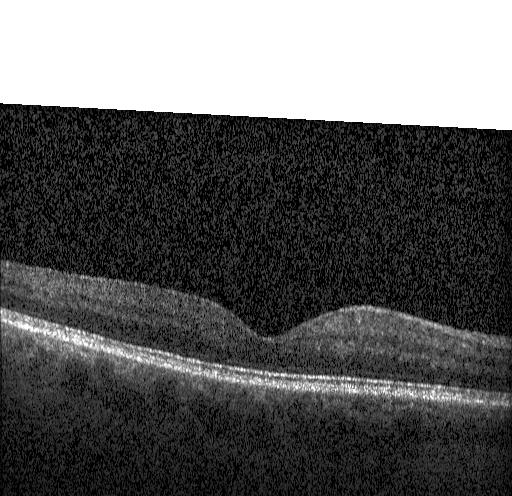 Horizontal scan through the fovea; retinal OCT B-scan; Heidelberg Spectralis; spectral-domain optical coherence tomography. OCT finding: no choroidal neovascularization, no diabetic macular edema, and no drusen.